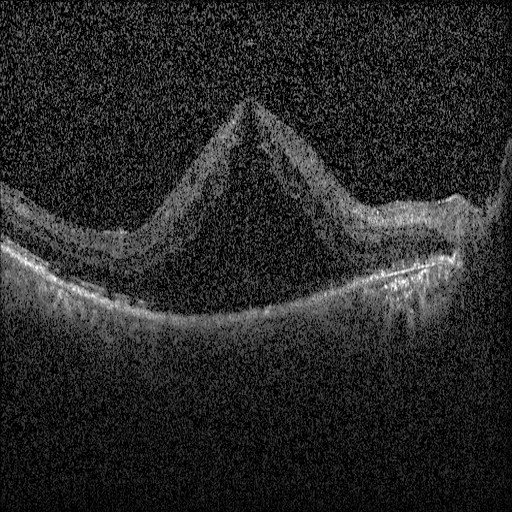

OCT B-scan.
Diabetic macular edema (DME).